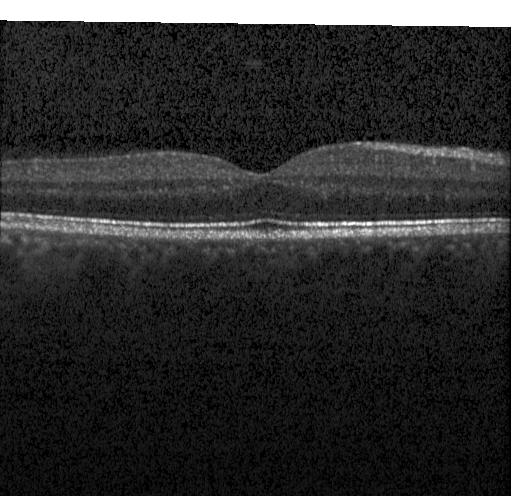 Retinal OCT cross-section — Dx: no evidence of choroidal neovascularization, diabetic macular edema, or drusen.